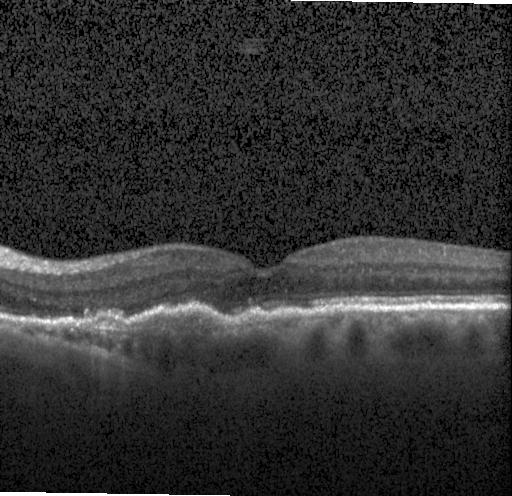 Finding: a choroidal neovascular membrane.